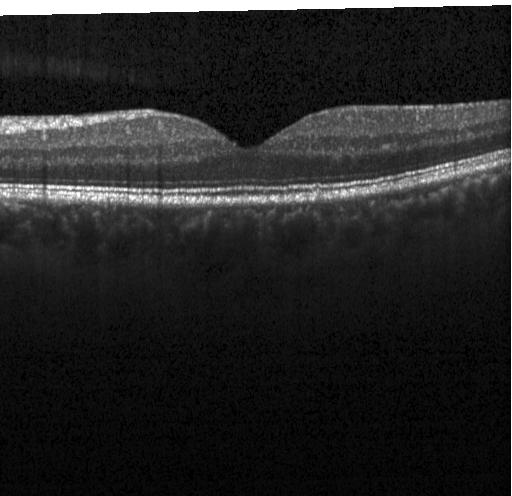 OCT line scan; Heidelberg Spectralis OCT system; spectral-domain OCT; through the macula — No choroidal neovascularization, no diabetic macular edema, and no drusen.